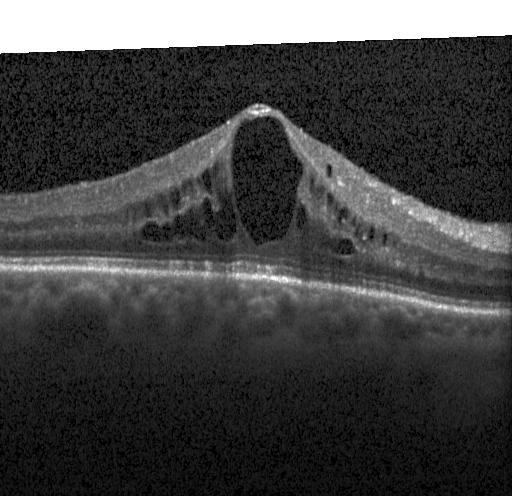
Retinal OCT cross-section; macular scan.
The scan shows diabetic macular edema.